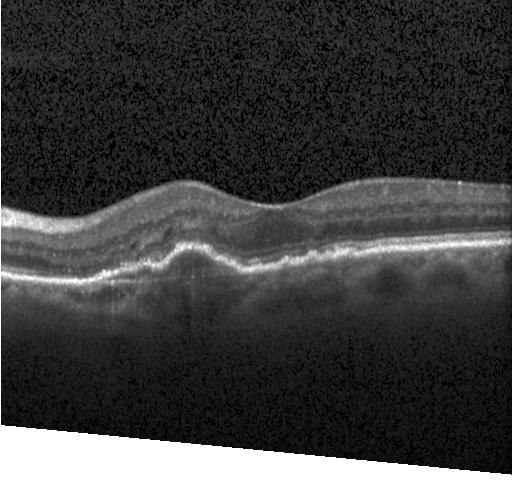 Macular scan; retinal OCT B-scan; spectral-domain optical coherence tomography.
Diagnosis: CNV.